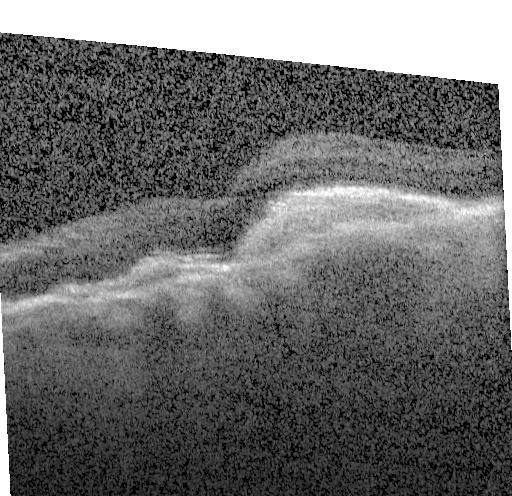 Acquired on a Heidelberg Spectralis; centered on the fovea; OCT B-scan
Macular OCT: choroidal neovascularization.